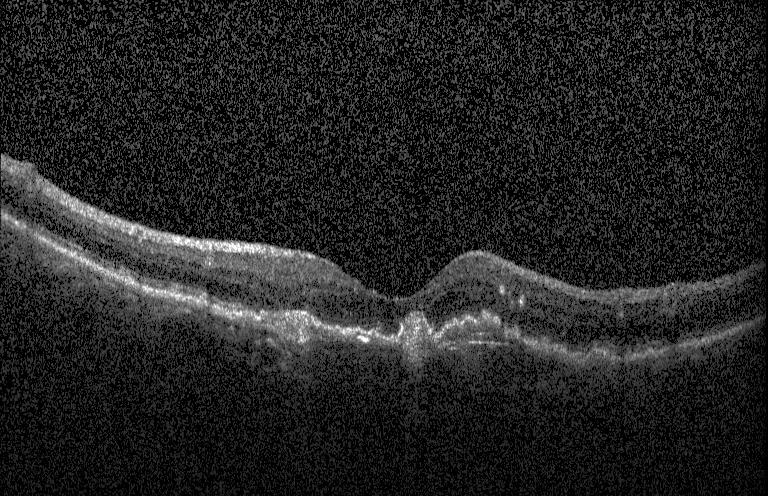
Optical coherence tomography scan
This B-scan demonstrates a choroidal neovascular membrane.